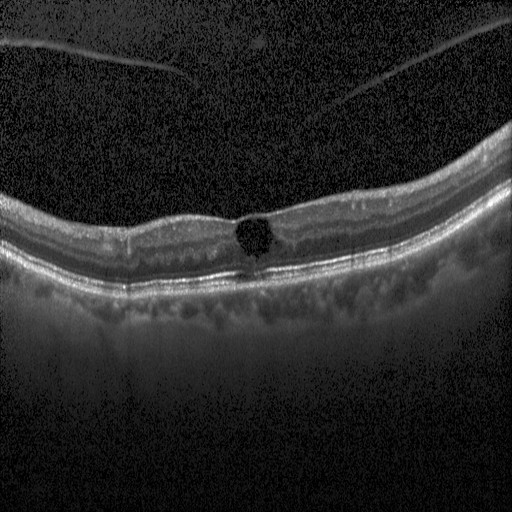 Optical coherence tomography B-scan; spectral-domain OCT.
Diagnosis: DME.